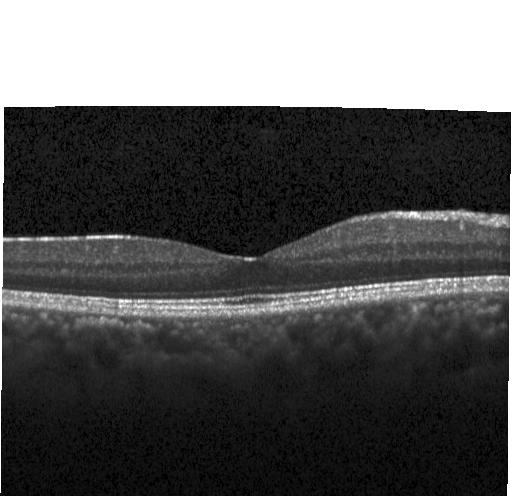
Instrument: Heidelberg Spectralis; optical coherence tomography B-scan; fovea-centered — Finding: neither choroidal neovascularization, diabetic macular edema, nor drusen.